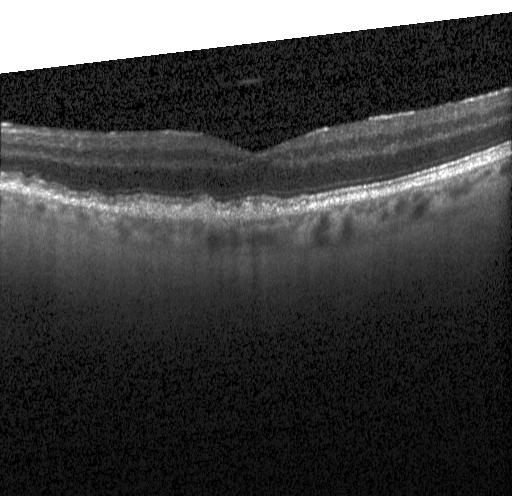 Spectral-domain OCT B-scan: multiple drusen.